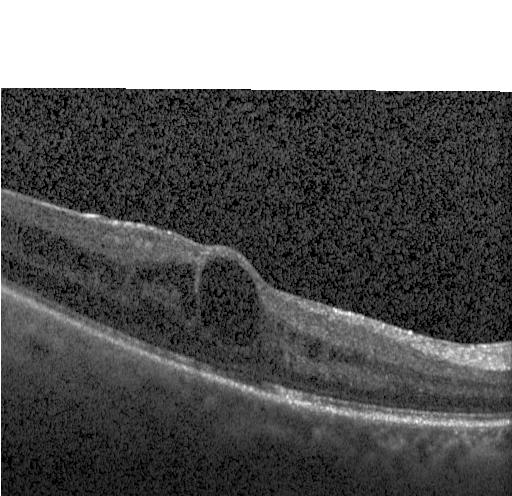 Retinal OCT B-scan. Heidelberg Spectralis. Spectral-domain optical coherence tomography — DME.